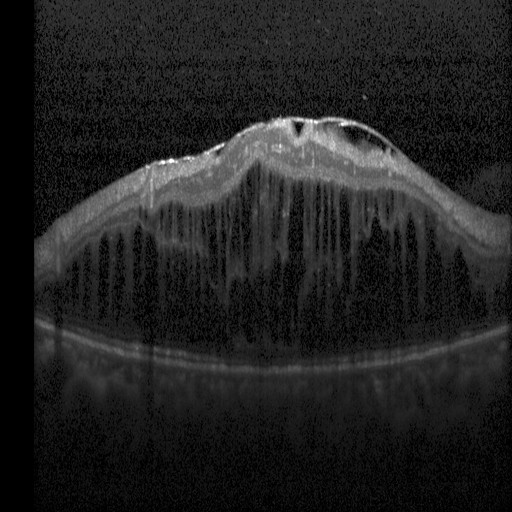

This B-scan demonstrates DME.